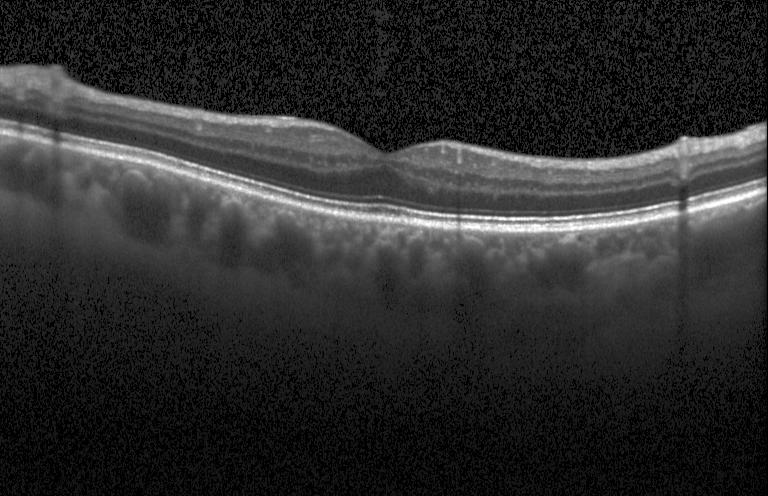
Acquired on a Heidelberg Spectralis, retinal OCT cross-section, macular scan. Impression: no choroidal neovascularization, diabetic macular edema, or drusen.